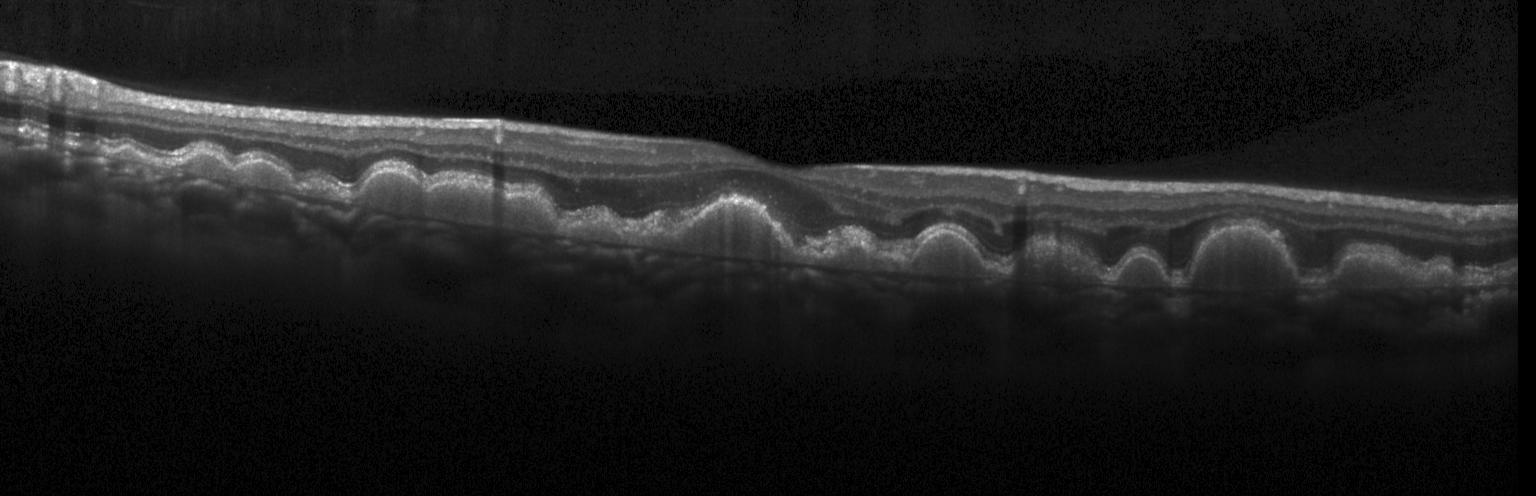 OCT B-scan — OCT finding: drusen.